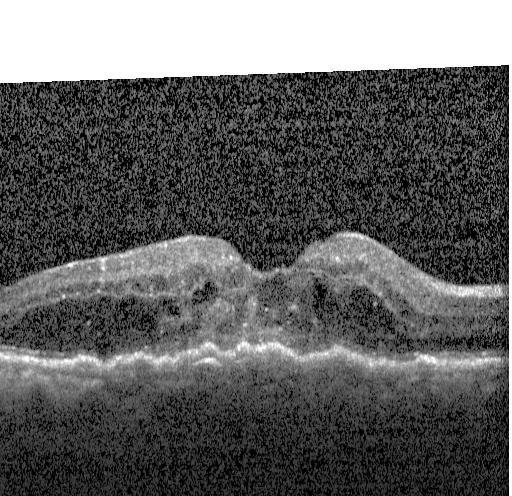

Finding: a choroidal neovascular membrane.